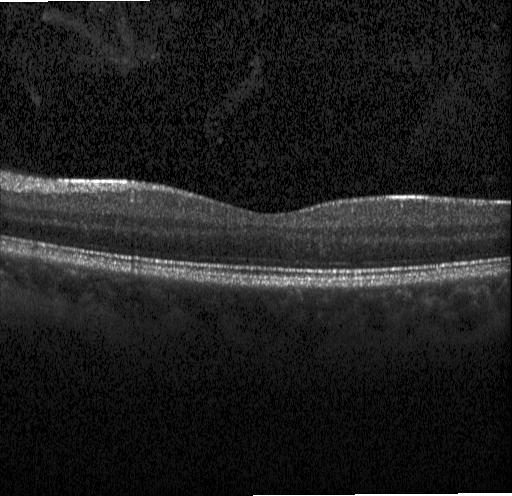 Acquired on a Heidelberg Spectralis, OCT line scan
Finding: neither CNV, DME, nor drusen.